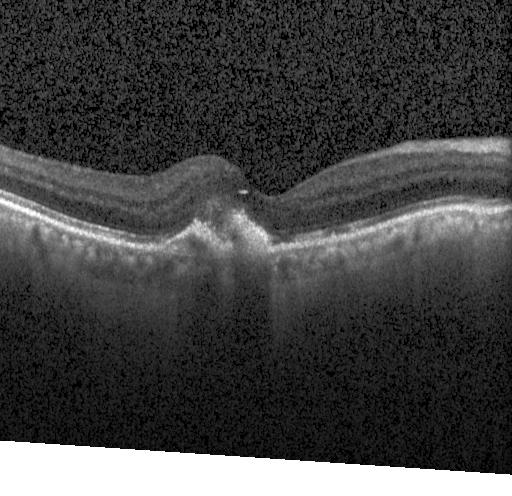

Impression: a choroidal neovascular membrane.